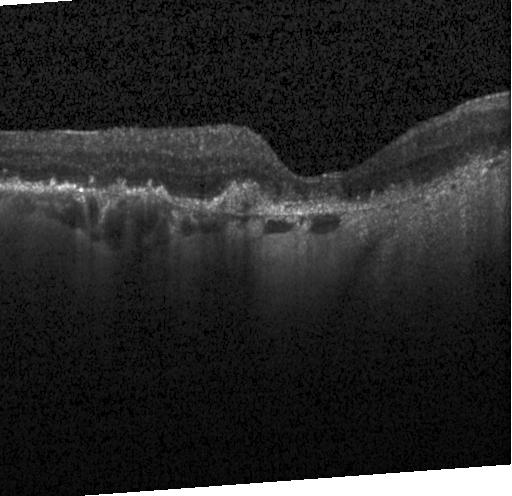 Heidelberg Spectralis OCT system · optical coherence tomography scan · SD-OCT
Impression: a choroidal neovascular membrane.